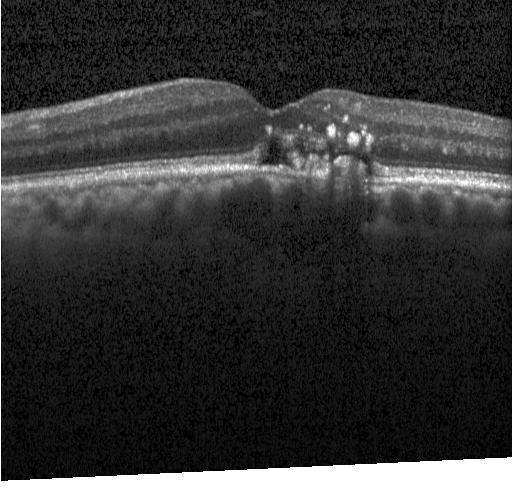

Optical coherence tomography scan; SD-OCT.
Assessment: a choroidal neovascular membrane.